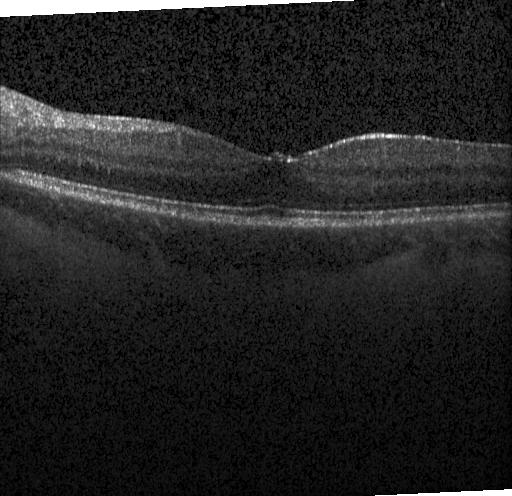

Through the macula · spectral-domain optical coherence tomography · retinal OCT cross-section · Heidelberg Spectralis OCT system.
Diagnosis: no choroidal neovascularization, no diabetic macular edema, and no drusen.